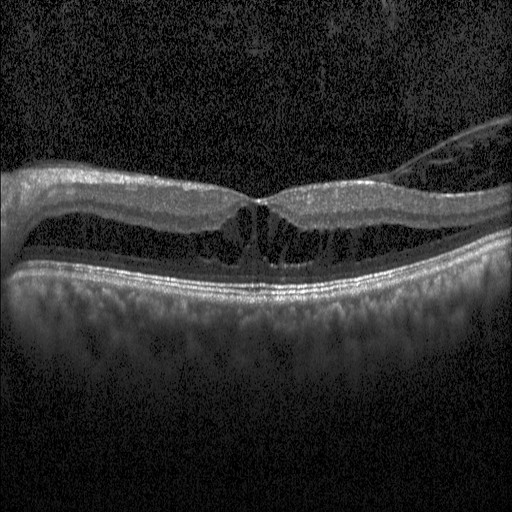
Diabetic macular edema (DME).